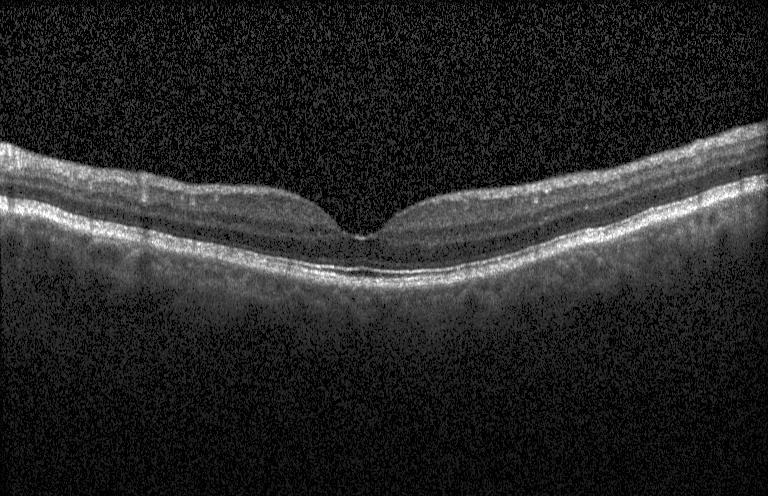
OCT line scan. Through the macula. Spectral-domain optical coherence tomography. Heidelberg Spectralis
Dx: no choroidal neovascularization, no diabetic macular edema, and no drusen.